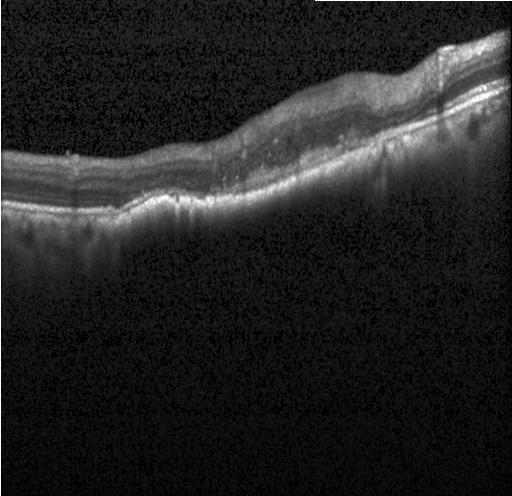

OCT line scan. Macular scan. Acquired on a Heidelberg Spectralis. Finding: a choroidal neovascular membrane.